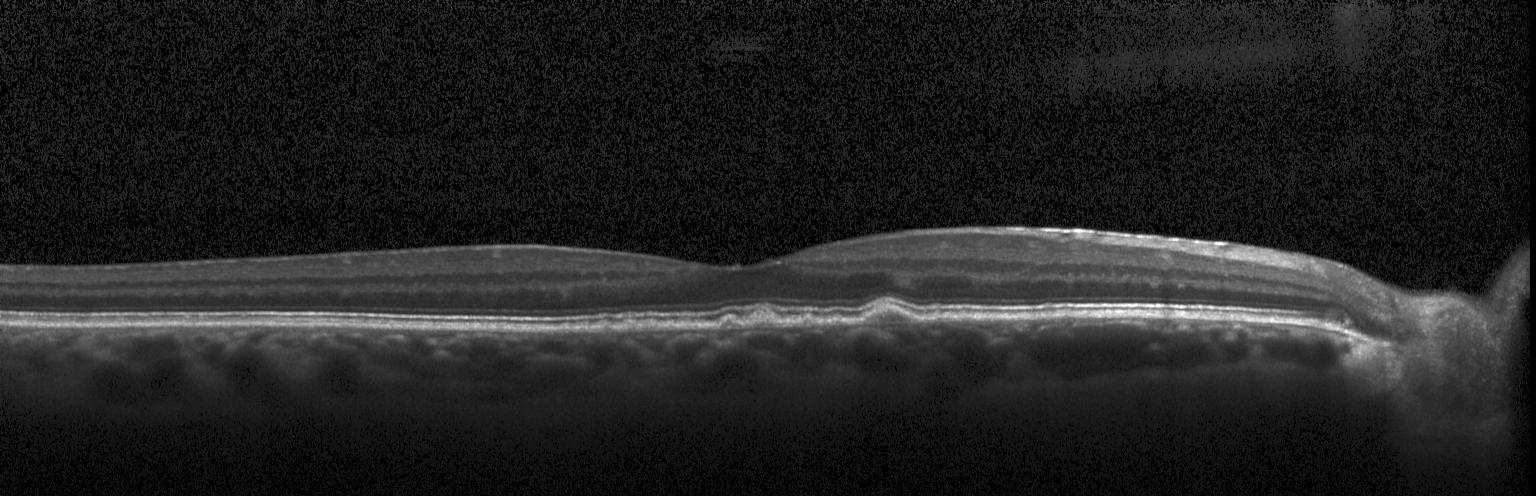 OCT line scan. Macular OCT: multiple drusen.